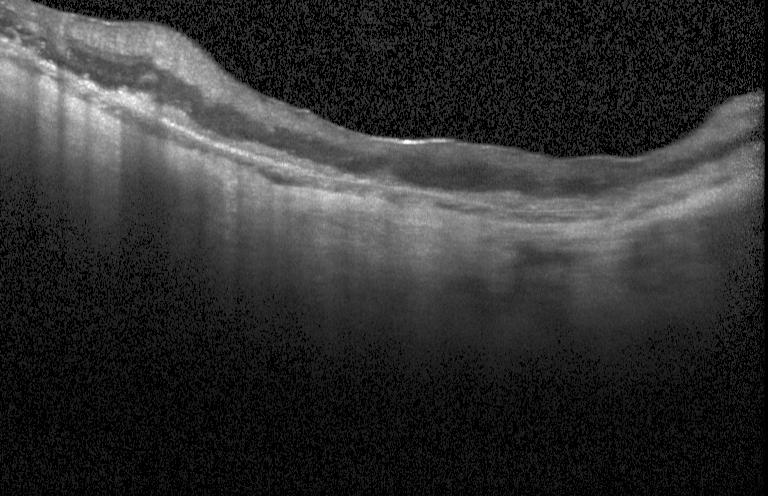

Heidelberg Spectralis; retinal OCT cross-section
The scan shows CNV.